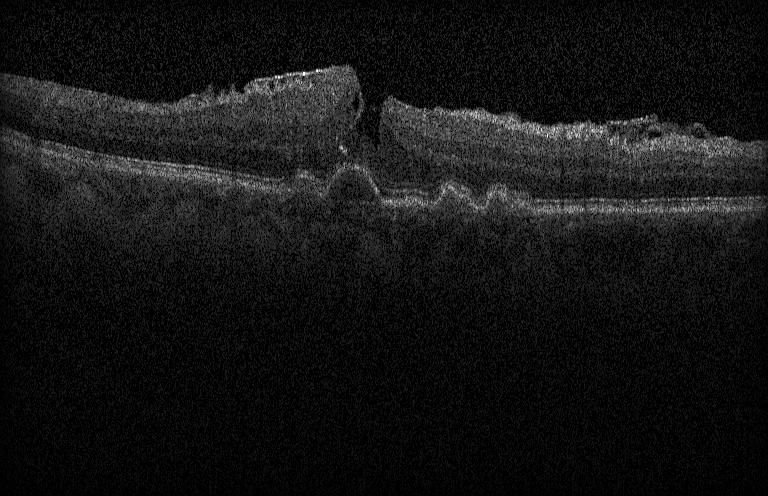

Centered on the fovea, retinal OCT cross-section, Heidelberg Spectralis.
The scan shows a choroidal neovascular membrane.